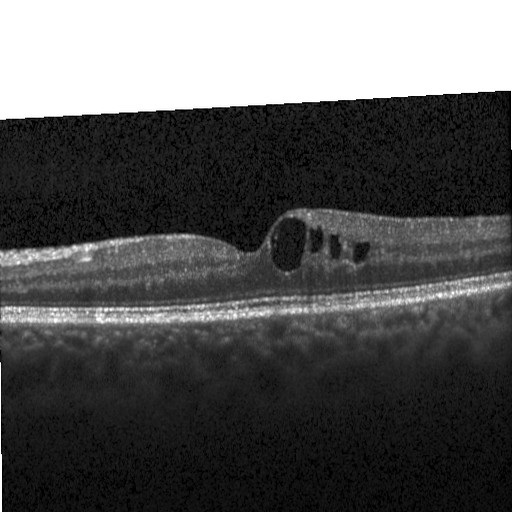
Spectral-domain optical coherence tomography, horizontal scan through the fovea, OCT line scan, Heidelberg Spectralis OCT system. Dx: diabetic macular edema.